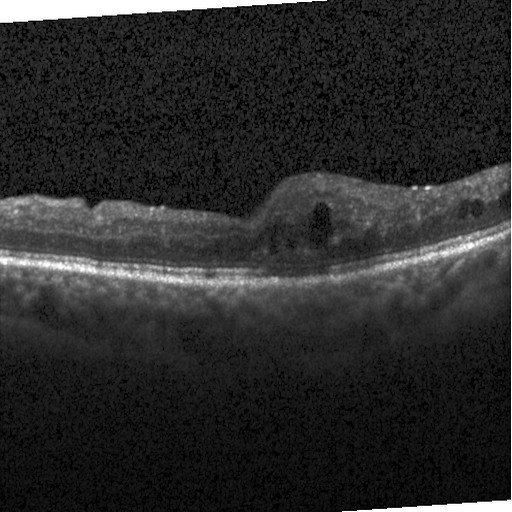

Horizontal scan through the fovea, Heidelberg Spectralis OCT system, optical coherence tomography B-scan, spectral-domain OCT. Assessment: DME.